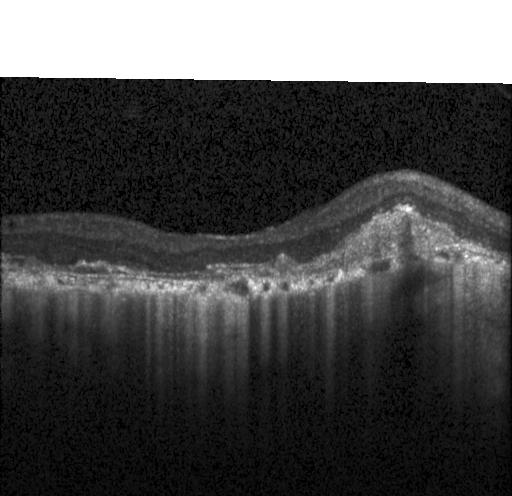 Spectral-domain optical coherence tomography · OCT B-scan · Heidelberg Spectralis OCT system. Finding: CNV.